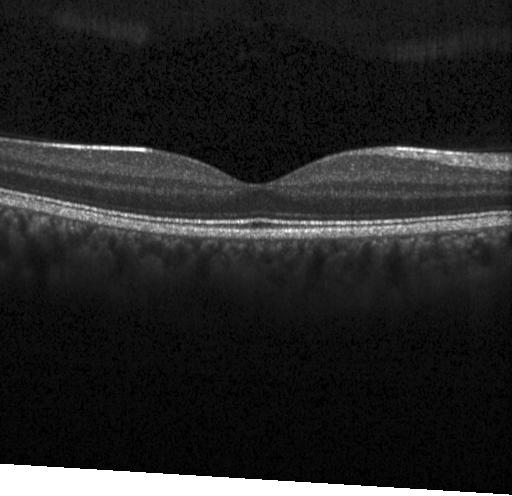

Spectral-domain optical coherence tomography, optical coherence tomography scan
The scan shows no evidence of choroidal neovascularization, diabetic macular edema, or drusen.